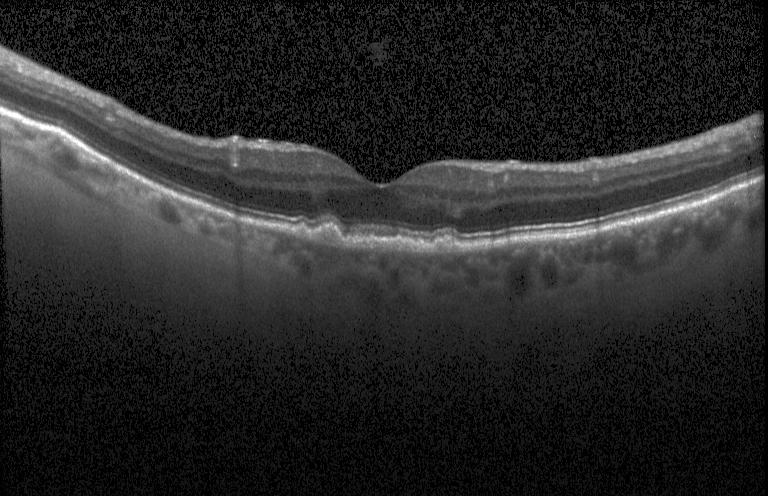

Optical coherence tomography B-scan
The scan shows sub-RPE drusenoid deposits.